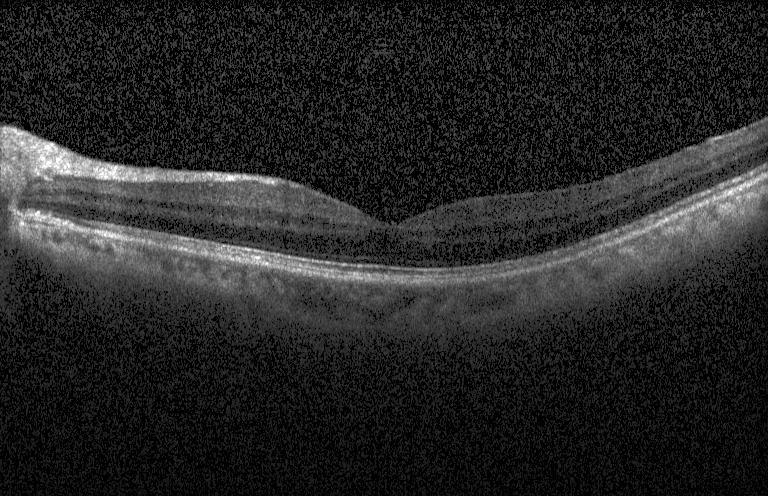 Retinal OCT B-scan; instrument: Heidelberg Spectralis.
Finding: no evidence of choroidal neovascularization, diabetic macular edema, or drusen.